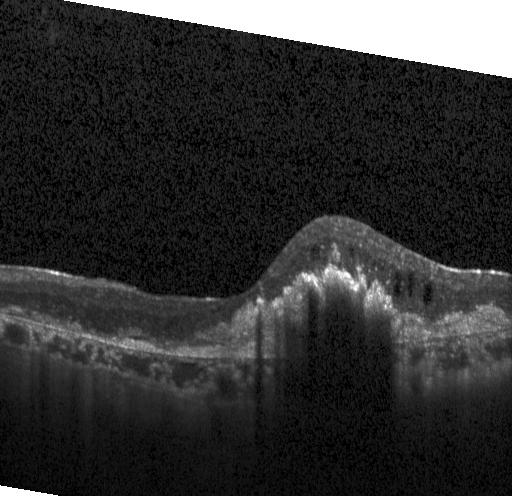
OCT B-scan, acquired on a Heidelberg Spectralis
Finding: CNV.